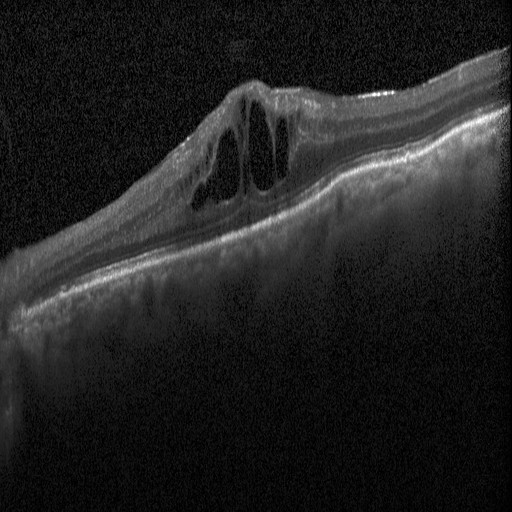 OCT B-scan. Horizontal scan through the fovea. Heidelberg Spectralis. Spectral-domain optical coherence tomography
Diagnosis: diabetic macular edema (DME).